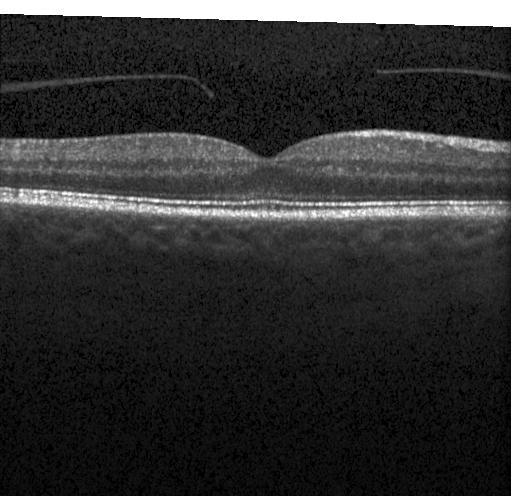
No choroidal neovascularization, diabetic macular edema, or drusen.